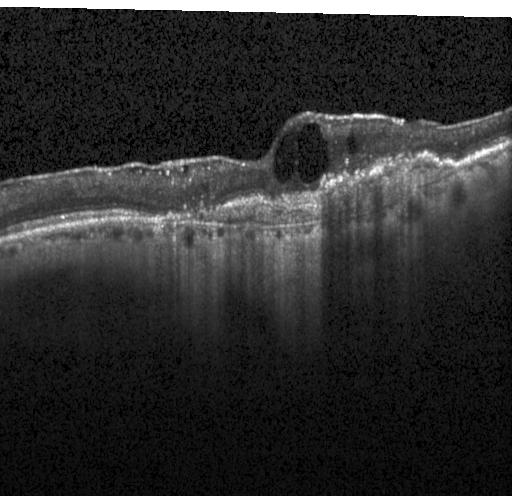
Optical coherence tomography B-scan — This B-scan demonstrates choroidal neovascularization (CNV).